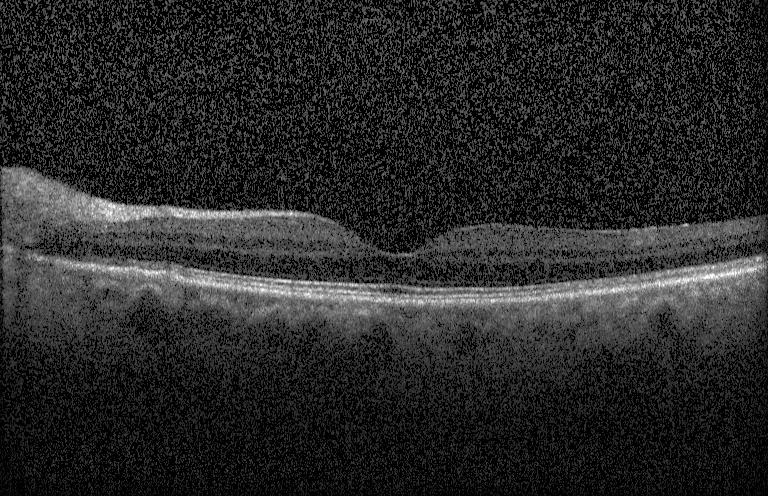
SD-OCT, fovea-centered, OCT B-scan. The scan shows no choroidal neovascularization, diabetic macular edema, or drusen.